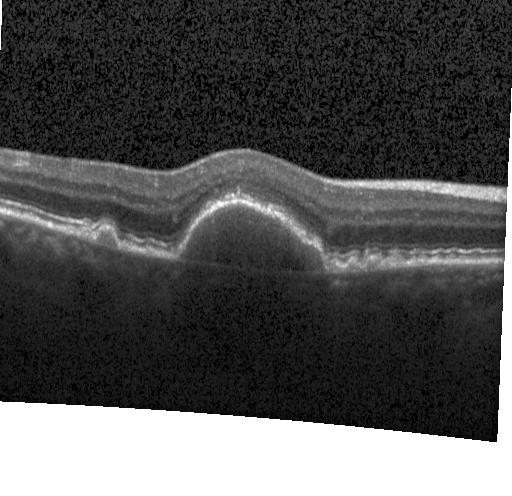

Instrument: Heidelberg Spectralis, retinal OCT cross-section, fovea-centered, spectral-domain optical coherence tomography — Finding: a choroidal neovascular membrane.